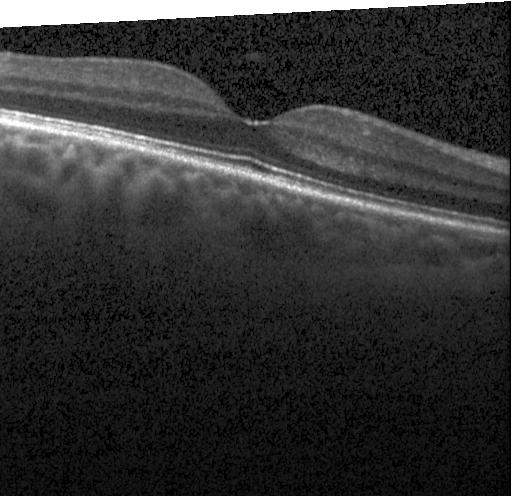
Spectral-domain OCT; Heidelberg Spectralis OCT system; retinal OCT cross-section — Assessment: no CNV, no DME, and no drusen.